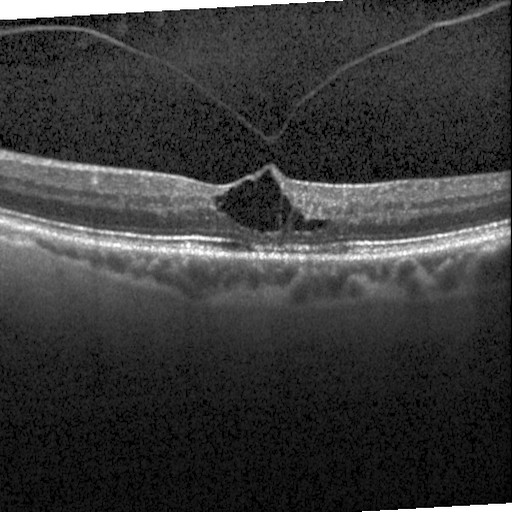 OCT B-scan · spectral-domain optical coherence tomography.
Finding: DME.